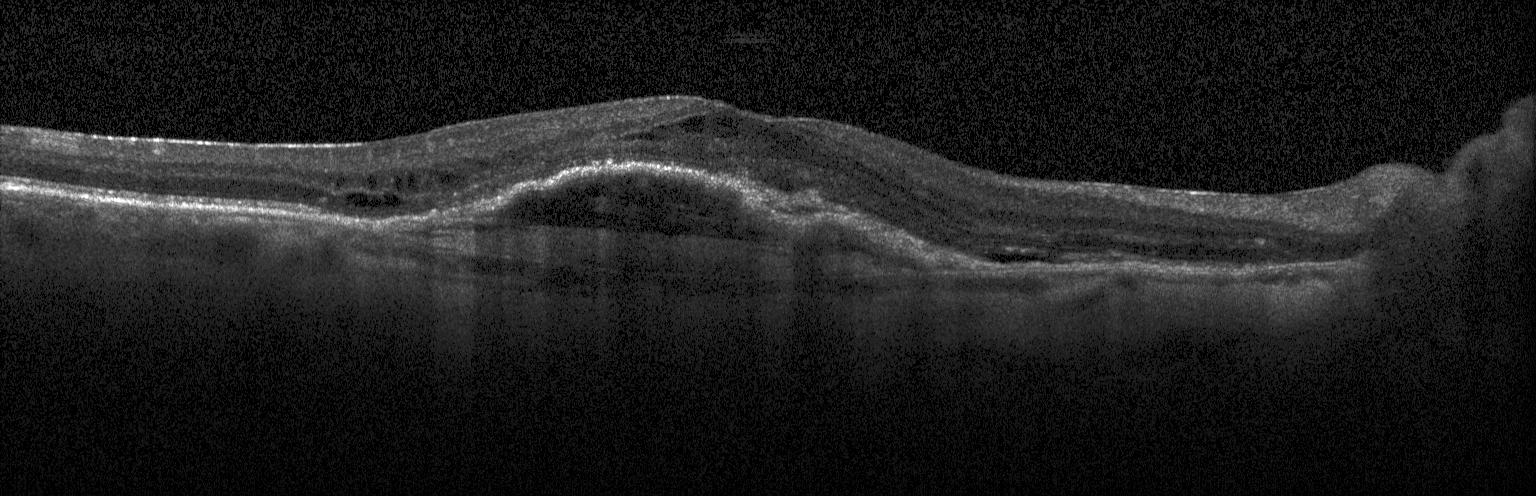

Optical coherence tomography B-scan, SD-OCT, centered on the fovea.
Assessment: a choroidal neovascular membrane.